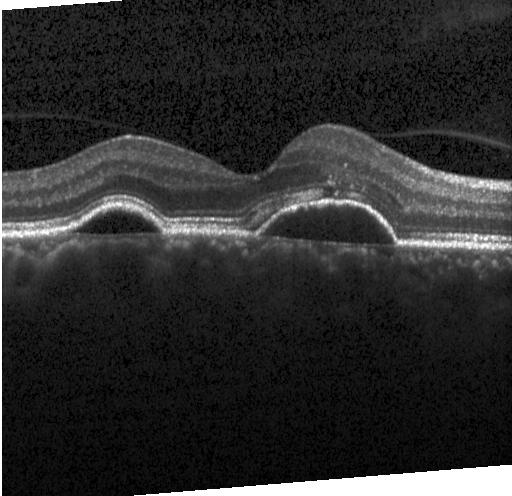
Macular OCT demonstrating choroidal neovascularization.